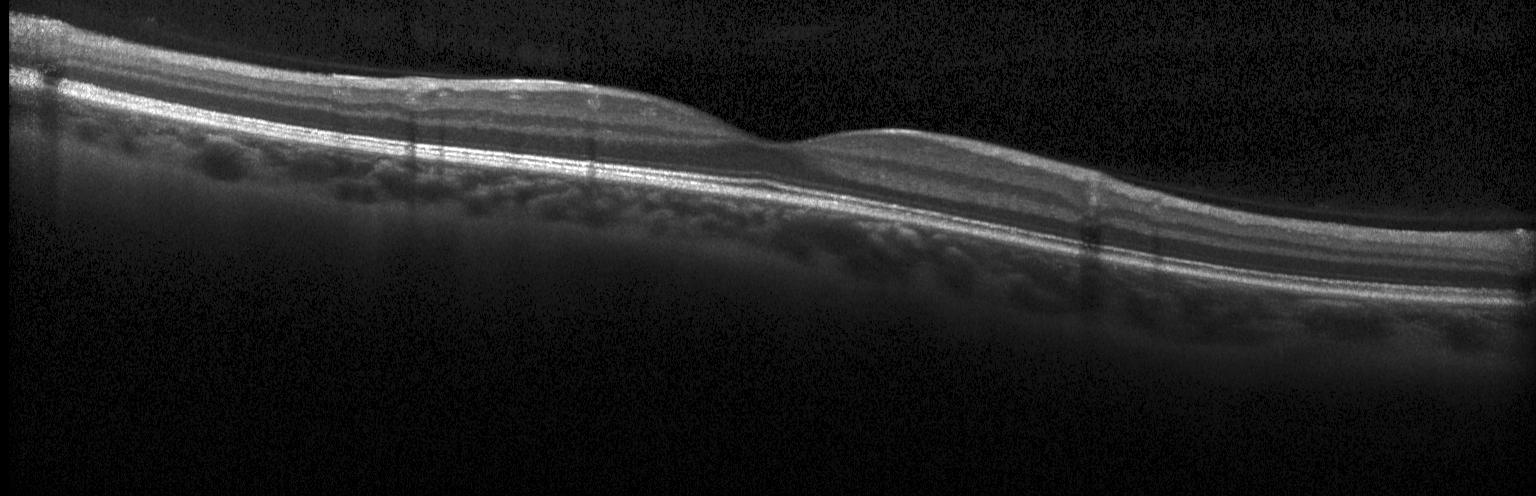 Optical coherence tomography scan; spectral-domain optical coherence tomography
Dx: neither CNV, DME, nor drusen.